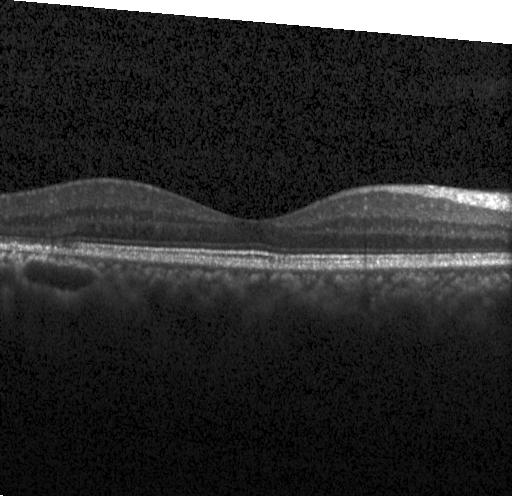

Macular OCT: no choroidal neovascularization, diabetic macular edema, or drusen.